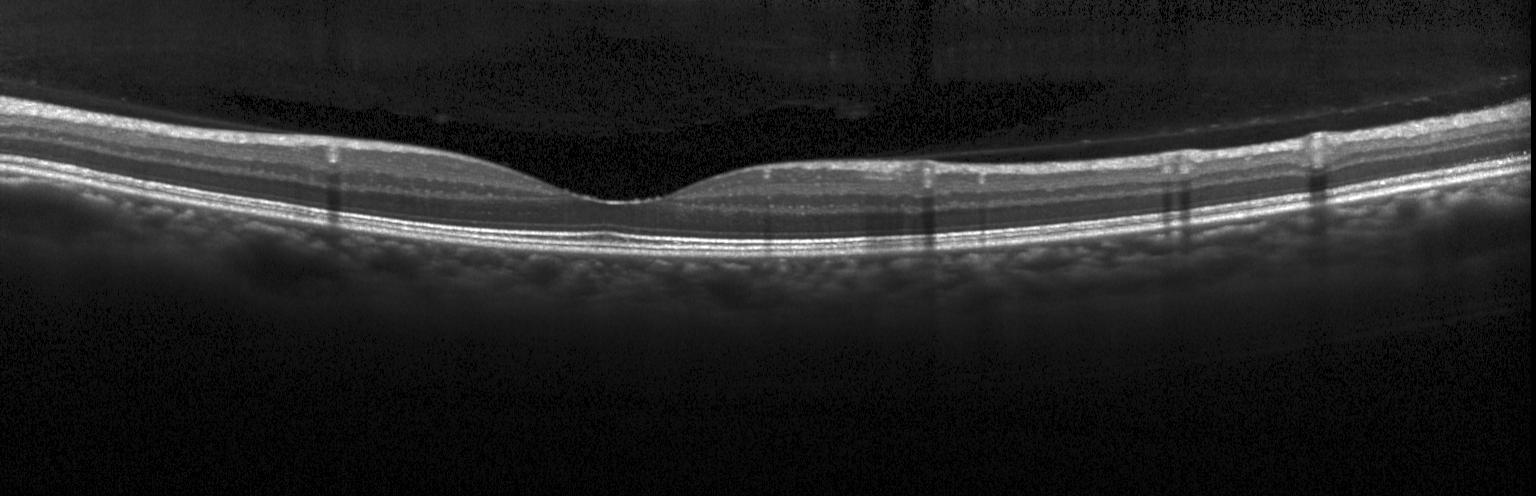

OCT line scan; Heidelberg Spectralis. Impression: no choroidal neovascularization, diabetic macular edema, or drusen.